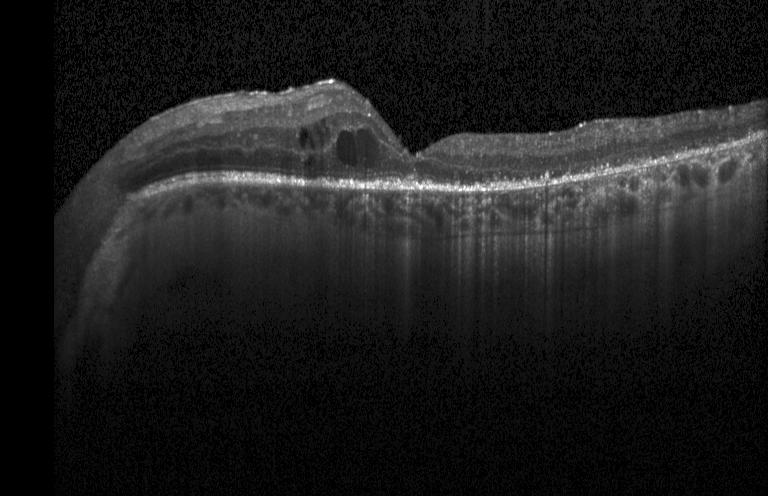

Through the macula, OCT B-scan, spectral-domain OCT, Heidelberg Spectralis OCT system. Finding: diabetic macular edema.